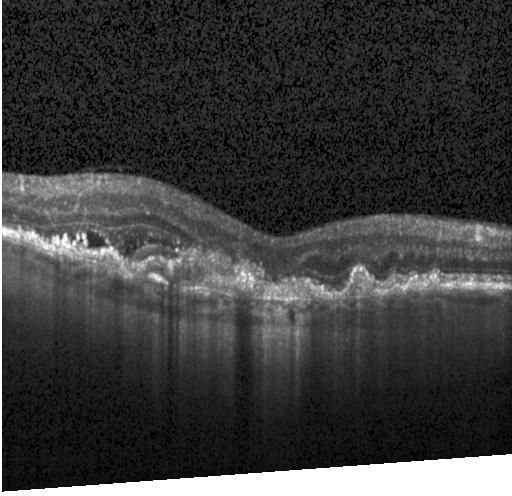 Heidelberg Spectralis OCT system, OCT B-scan, spectral-domain optical coherence tomography, macular scan.
This B-scan demonstrates choroidal neovascularization.